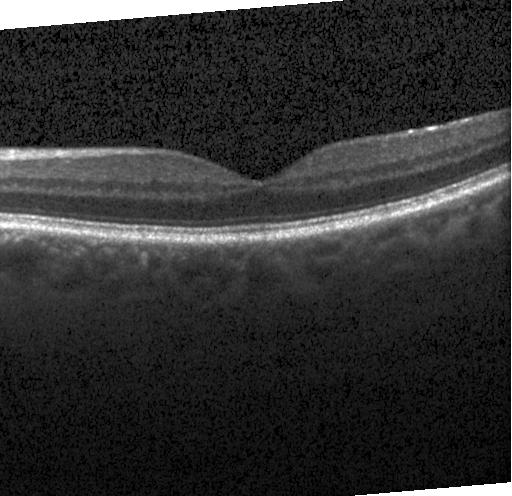

Retinal OCT cross-section; centered on the fovea; instrument: Heidelberg Spectralis — Impression: no evidence of choroidal neovascularization, diabetic macular edema, or drusen.